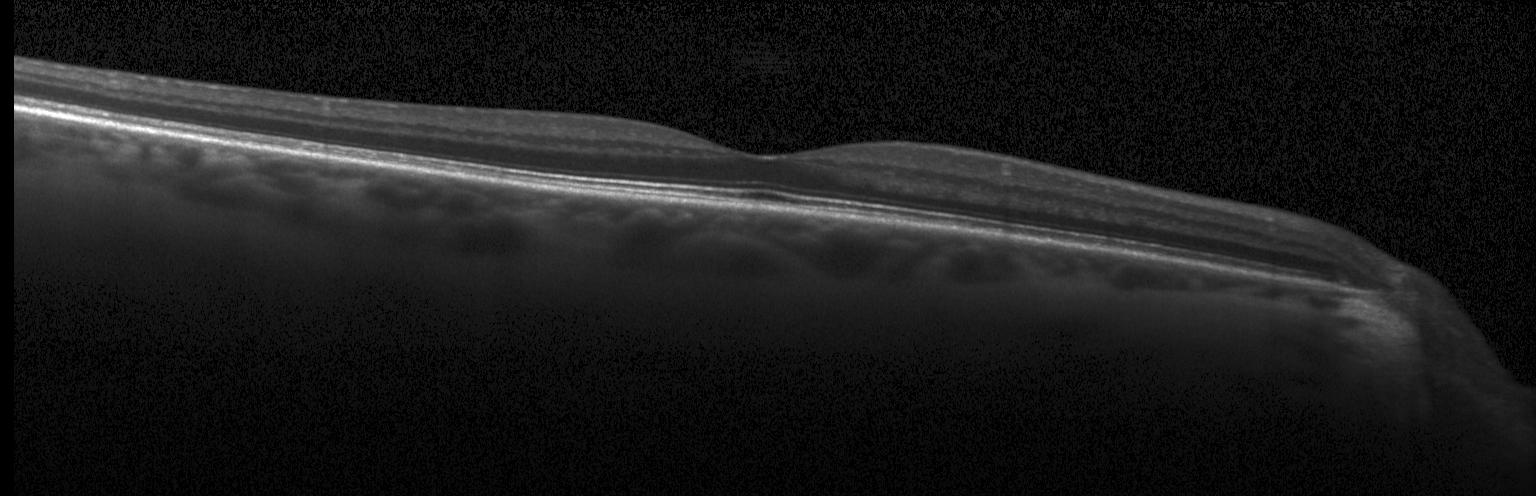 Centered on the fovea · OCT line scan. Neither choroidal neovascularization, diabetic macular edema, nor drusen.